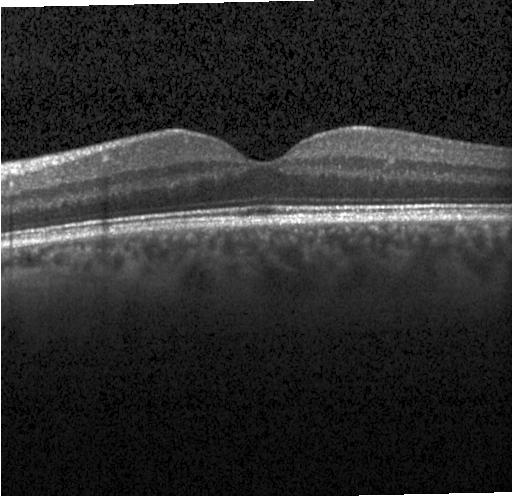 Heidelberg Spectralis; spectral-domain optical coherence tomography; macular scan; OCT line scan — Impression: neither CNV, DME, nor drusen.